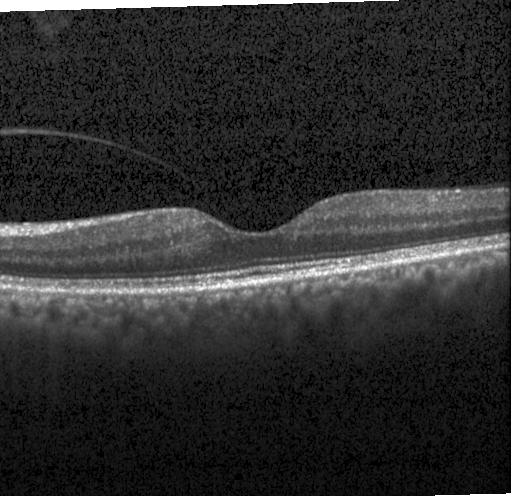

Spectral-domain optical coherence tomography. OCT line scan. Instrument: Heidelberg Spectralis — Impression: no evidence of choroidal neovascularization, diabetic macular edema, or drusen.